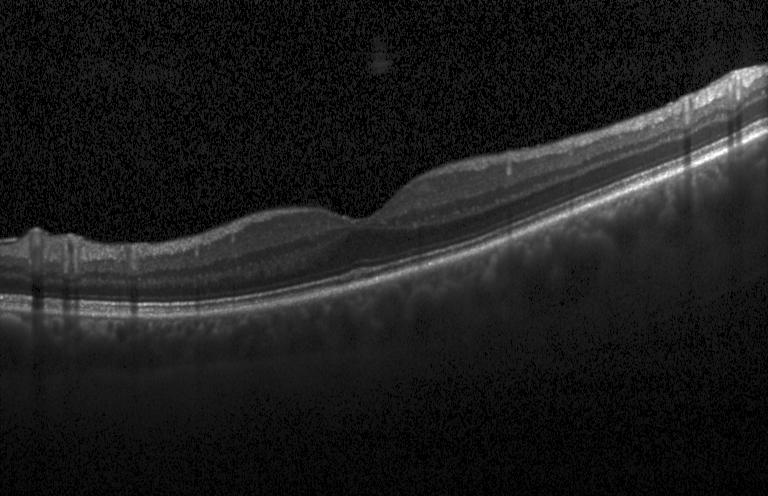
Spectral-domain optical coherence tomography, optical coherence tomography scan, Heidelberg Spectralis OCT system, through the macula — Diagnosis: no evidence of choroidal neovascularization, diabetic macular edema, or drusen.